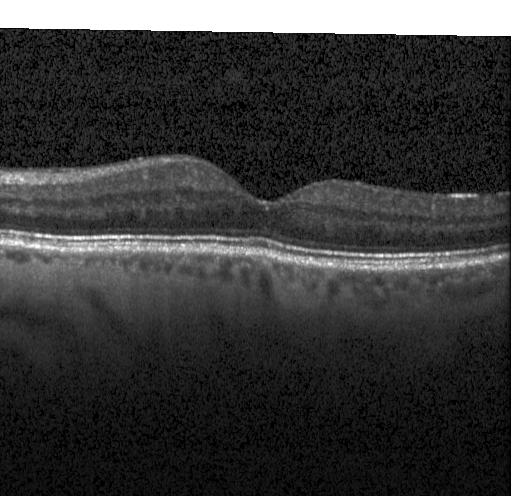
Fovea-centered. Spectral-domain OCT. Heidelberg Spectralis. Retinal OCT B-scan.
Dx: no choroidal neovascularization, diabetic macular edema, or drusen.